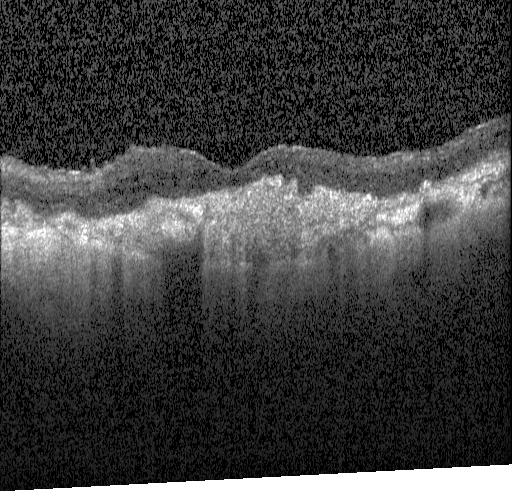 This B-scan demonstrates a choroidal neovascular membrane.